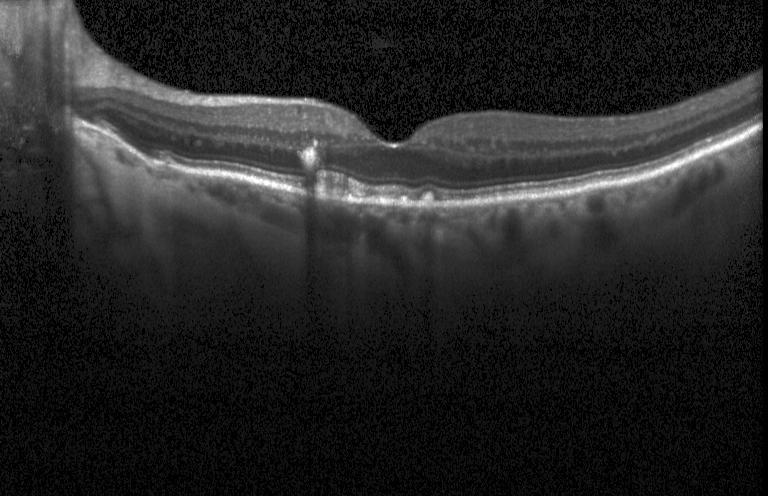

Retinal OCT cross-section
Assessment: sub-RPE drusenoid deposits.